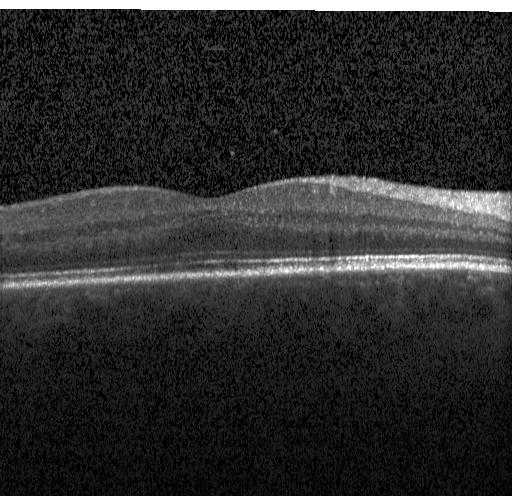
Spectral-domain OCT; Heidelberg Spectralis OCT system; retinal OCT cross-section. Dx: no choroidal neovascularization, no diabetic macular edema, and no drusen.